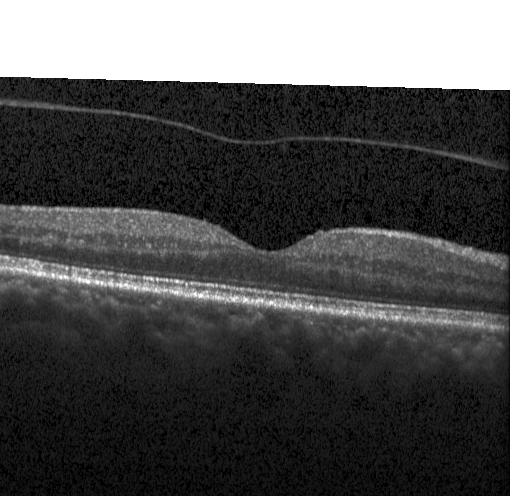
OCT B-scan, through the macula, instrument: Heidelberg Spectralis. The scan shows neither choroidal neovascularization, diabetic macular edema, nor drusen.